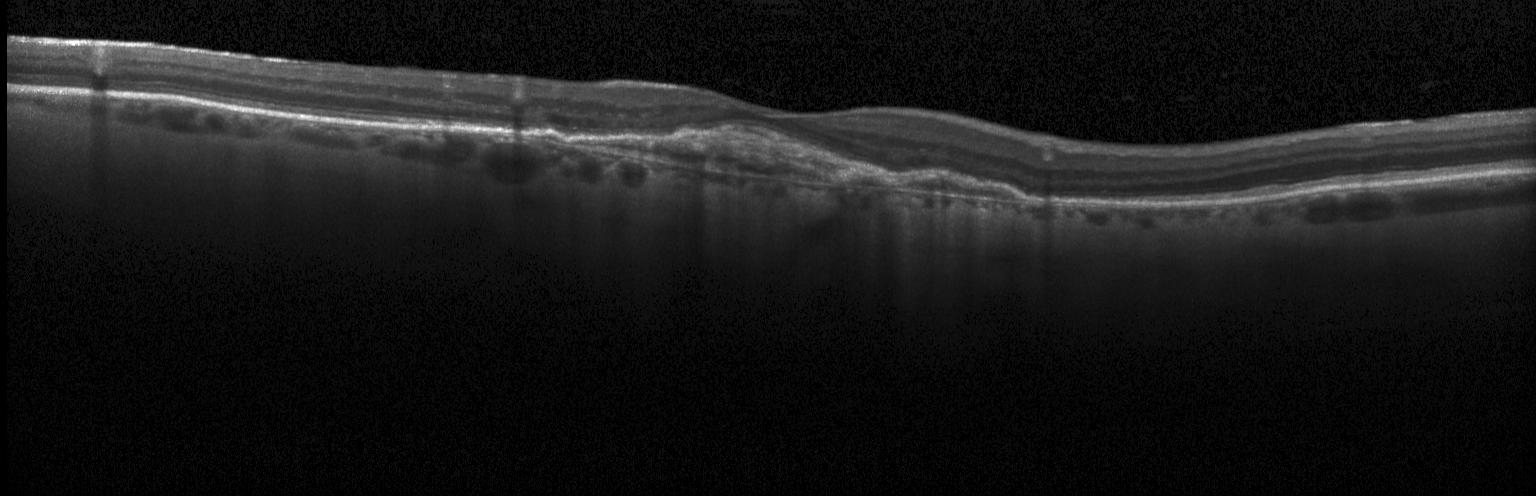

Retinal OCT B-scan; macular scan — Finding: CNV.